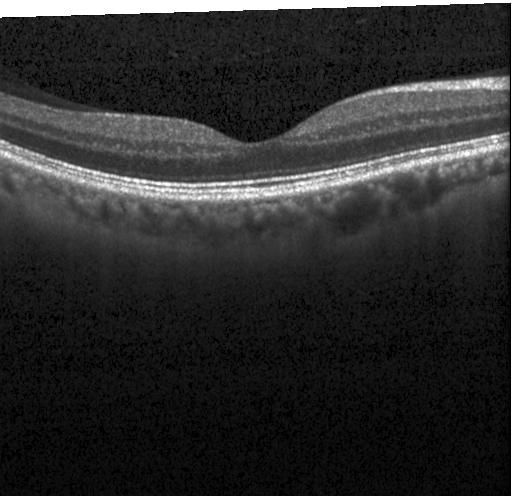

Optical coherence tomography scan, SD-OCT.
Impression: no choroidal neovascularization, no diabetic macular edema, and no drusen.